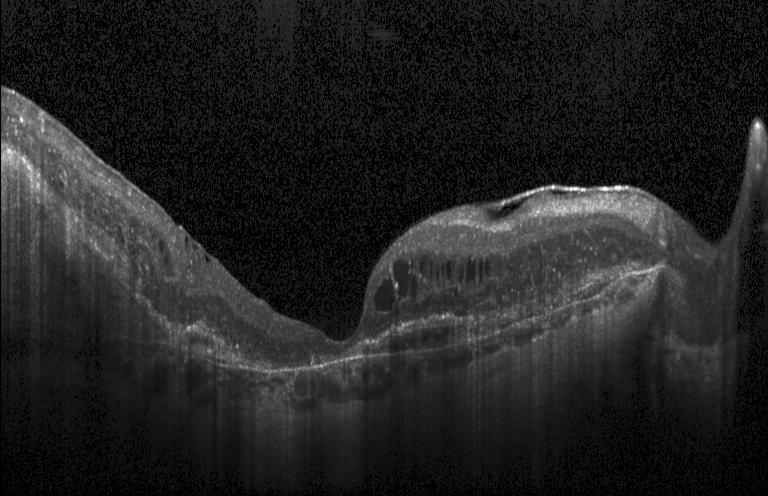 Instrument: Heidelberg Spectralis. Optical coherence tomography scan. SD-OCT — Impression: a choroidal neovascular membrane.